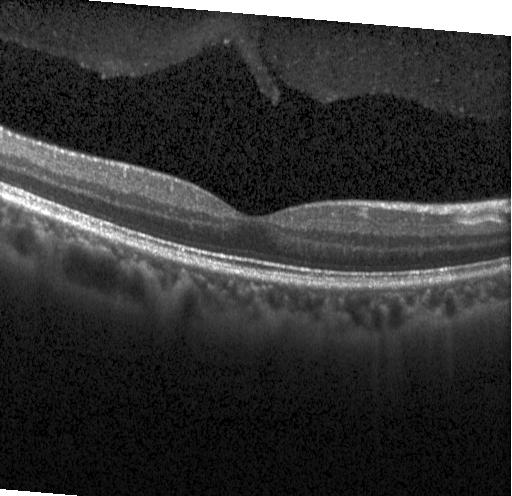

Retinal OCT cross-section.
Macular OCT: no CNV, DME, or drusen.